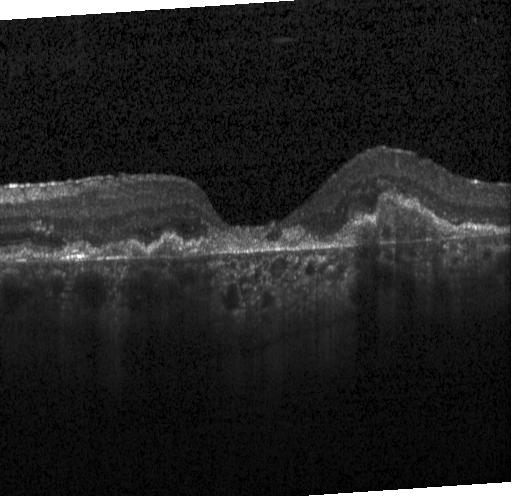 Optical coherence tomography scan
Assessment: a choroidal neovascular membrane.